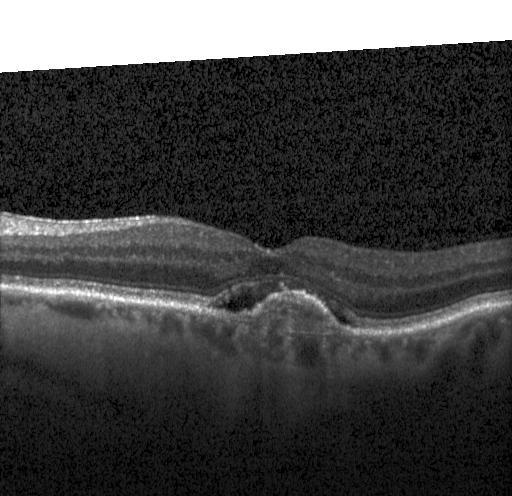
Spectral-domain optical coherence tomography; optical coherence tomography scan — Diagnosis: a choroidal neovascular membrane.